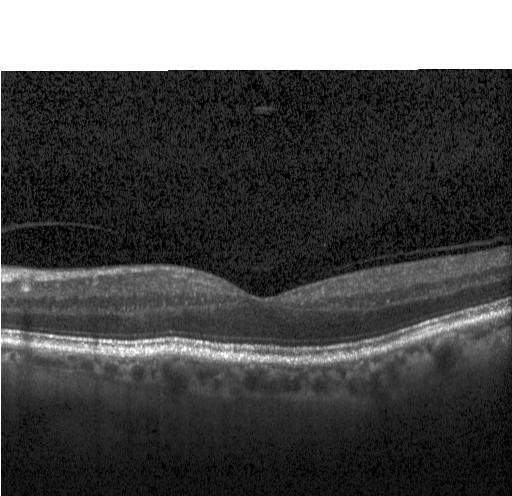

The scan shows no CNV, no DME, and no drusen.